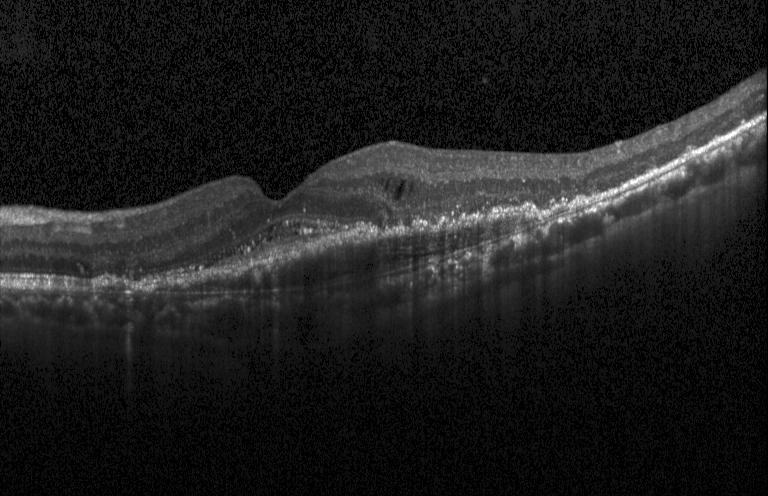
Spectral-domain OCT, retinal OCT B-scan. Impression: a choroidal neovascular membrane.